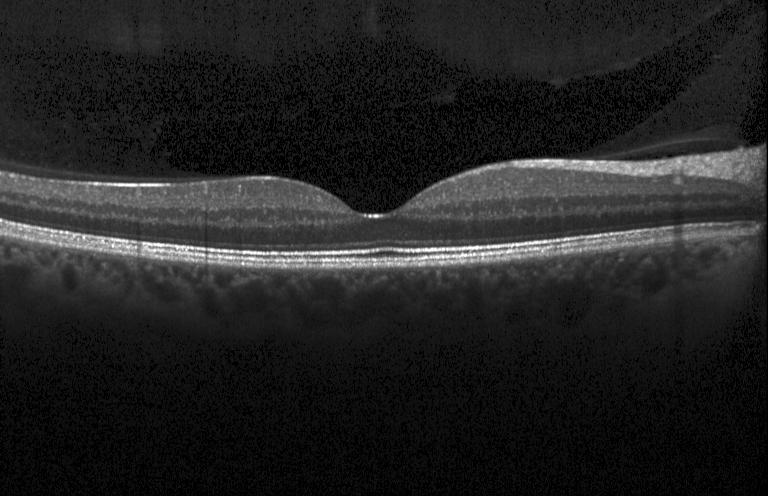 Horizontal scan through the fovea; OCT line scan; Heidelberg Spectralis
The scan shows no choroidal neovascularization, no diabetic macular edema, and no drusen.